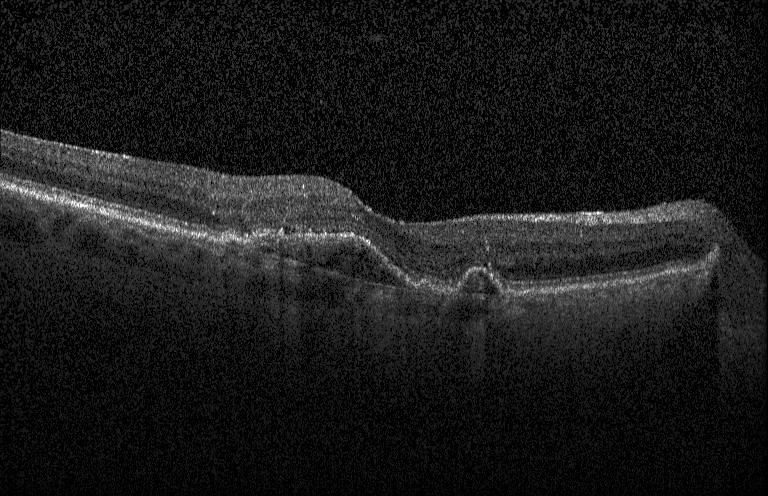
Dx: choroidal neovascularization (CNV).